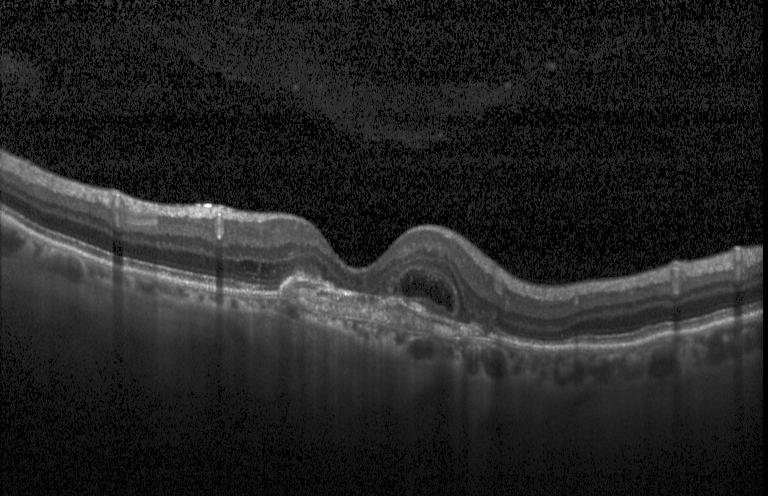

Fovea-centered · OCT B-scan.
Choroidal neovascularization.